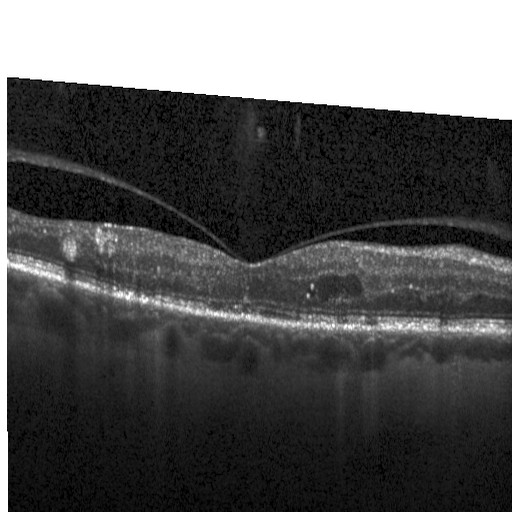
Macular scan · retinal OCT B-scan
DME.